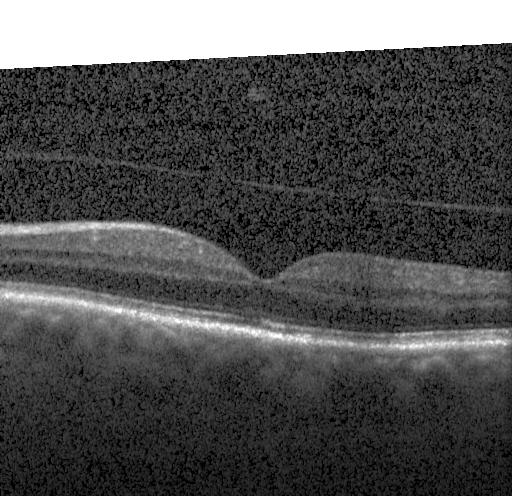

Finding: neither choroidal neovascularization, diabetic macular edema, nor drusen.